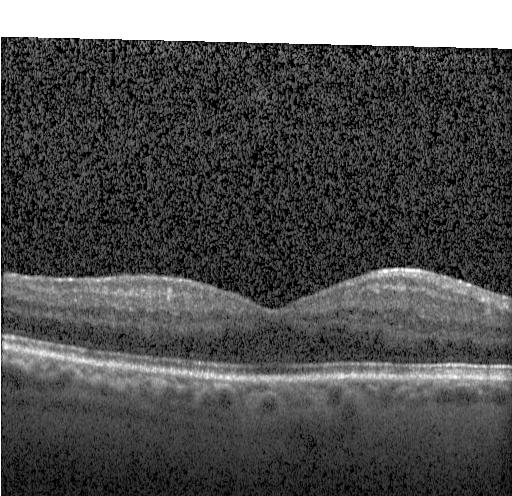 Spectral-domain OCT B-scan: no CNV, DME, or drusen.